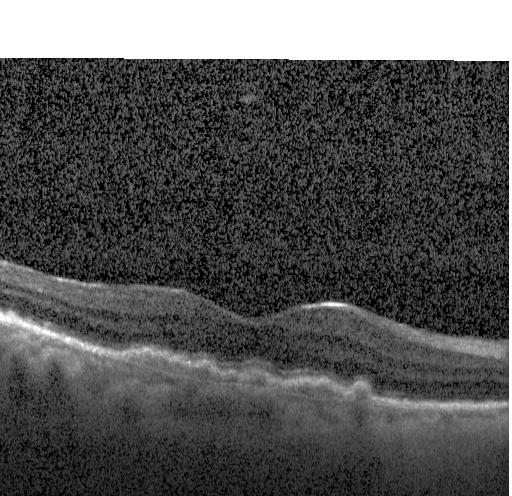
OCT B-scan
Diagnosis: a choroidal neovascular membrane.